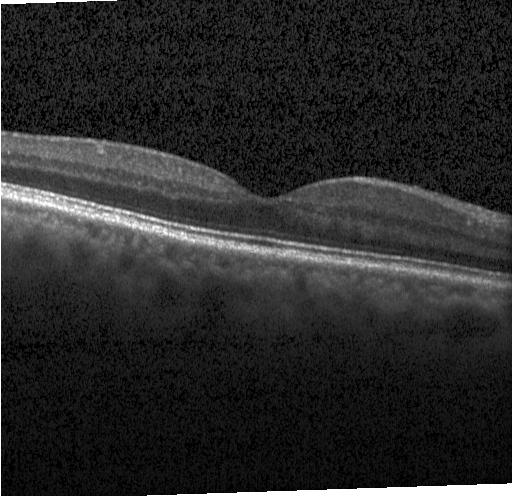

Spectral-domain optical coherence tomography, retinal OCT B-scan, through the macula, instrument: Heidelberg Spectralis — Finding: no choroidal neovascularization, diabetic macular edema, or drusen.